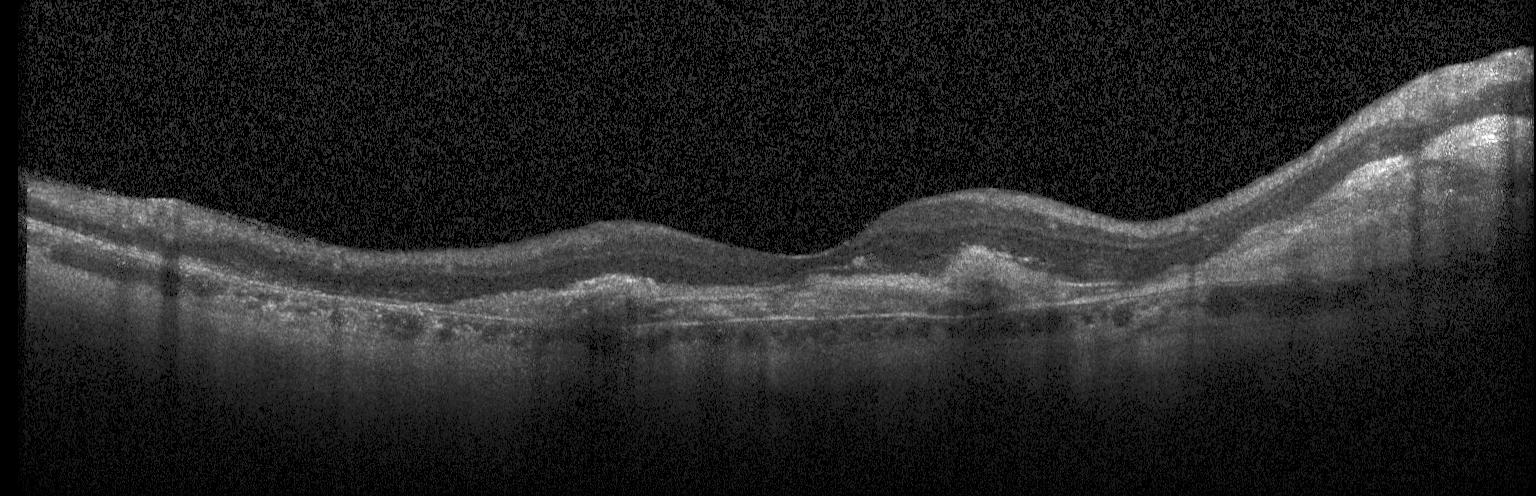

Dx: choroidal neovascularization.